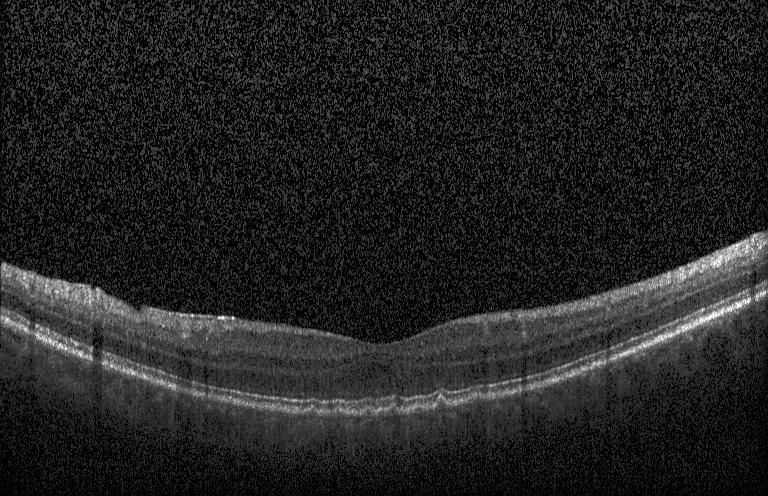
Spectral-domain optical coherence tomography, fovea-centered, optical coherence tomography B-scan.
Impression: multiple drusen.